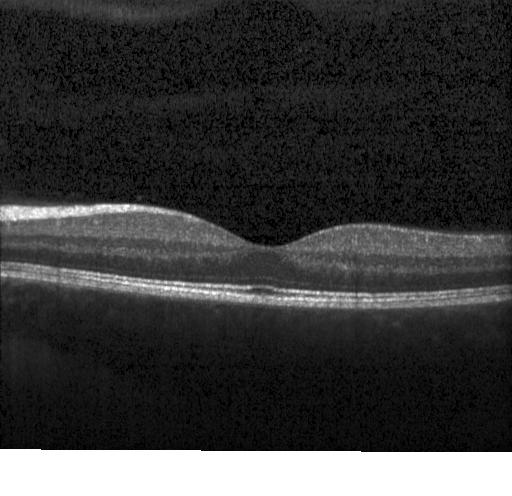 Finding: neither CNV, DME, nor drusen.